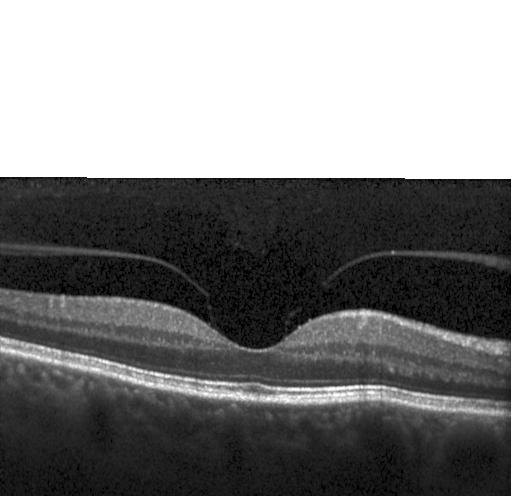

Finding: no choroidal neovascularization, no diabetic macular edema, and no drusen.